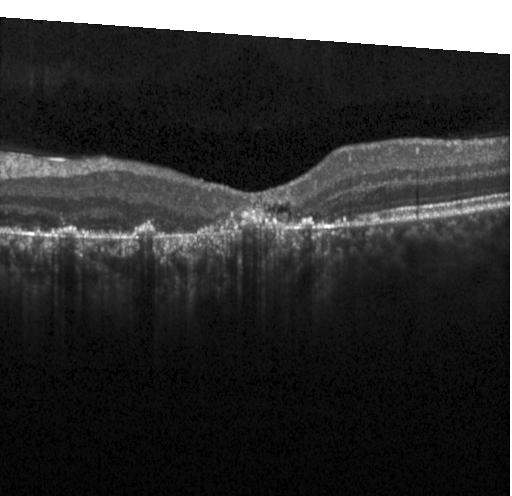 Retinal OCT B-scan
The scan shows CNV.